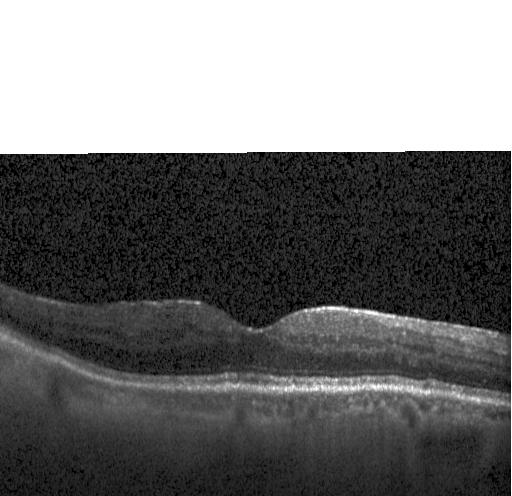

Impression: no choroidal neovascularization, no diabetic macular edema, and no drusen.